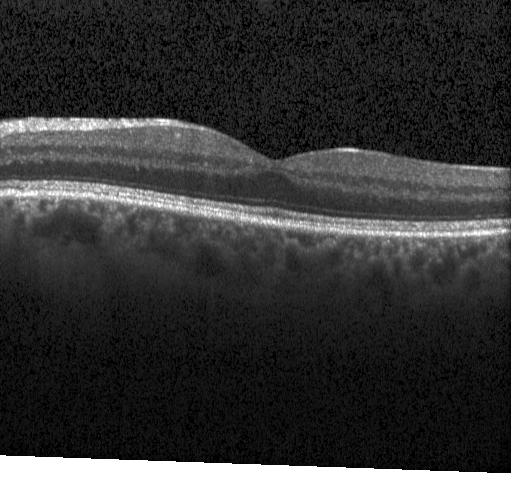
Instrument: Heidelberg Spectralis, optical coherence tomography scan, SD-OCT. Diagnosis: neither choroidal neovascularization, diabetic macular edema, nor drusen.